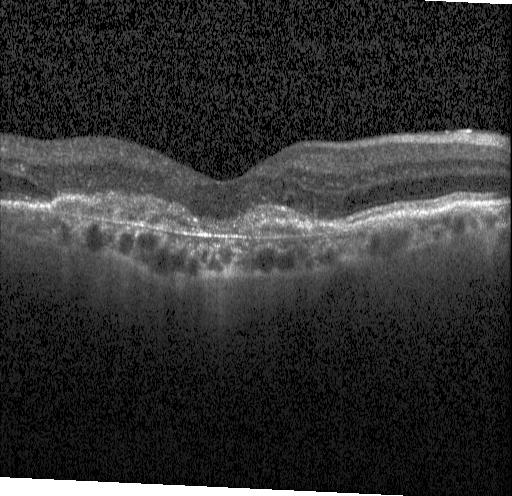

Optical coherence tomography B-scan. Fovea-centered
Dx: a choroidal neovascular membrane.